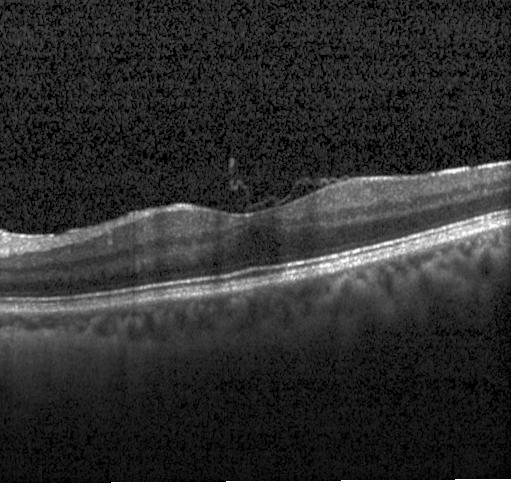 Impression: no choroidal neovascularization, no diabetic macular edema, and no drusen.